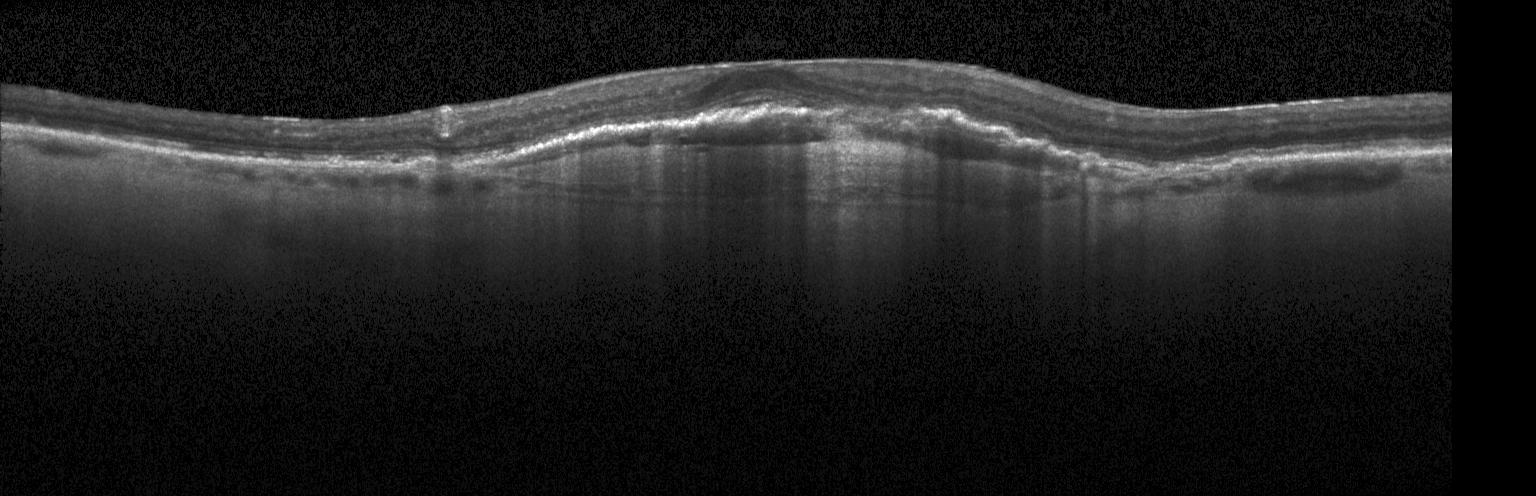
Retinal OCT B-scan. Through the macula. Impression: a choroidal neovascular membrane.